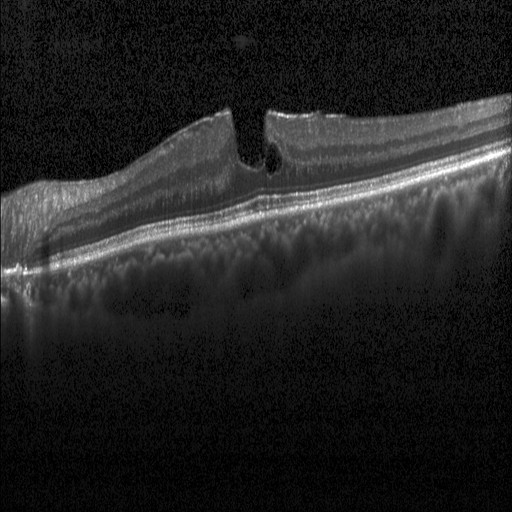 DME.